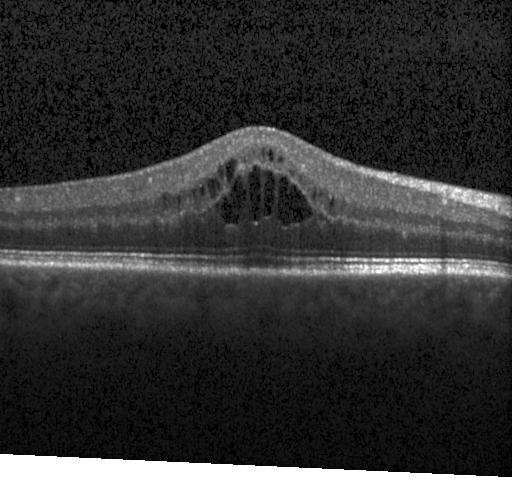 Impression: diabetic macular edema (DME).